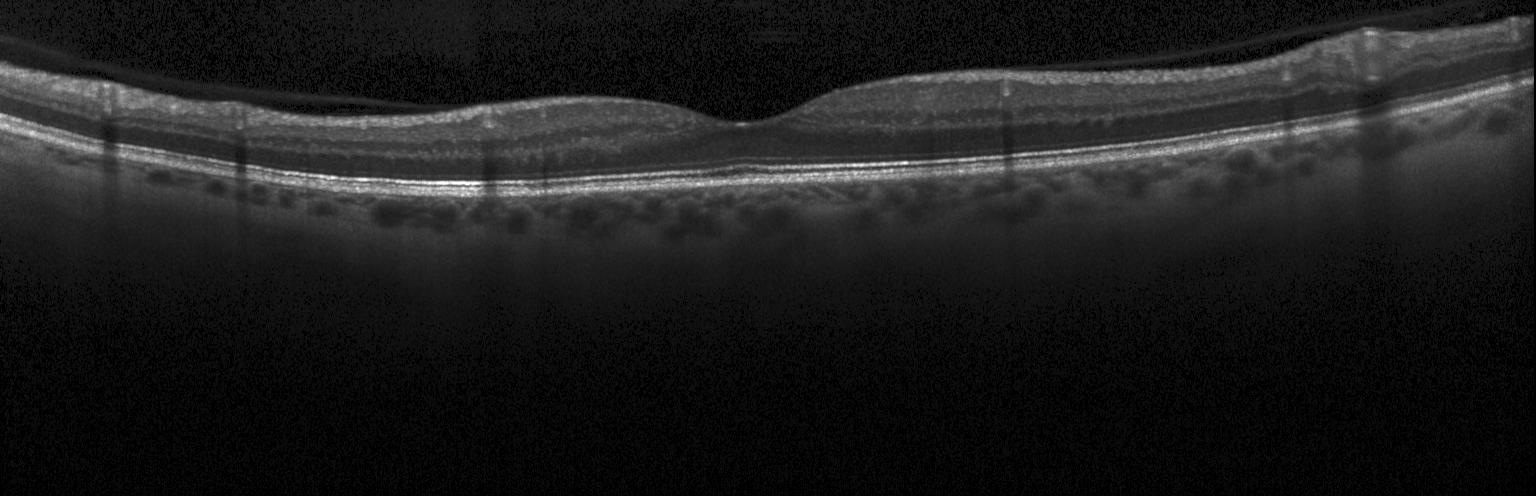

Finding: no evidence of CNV, DME, or drusen.